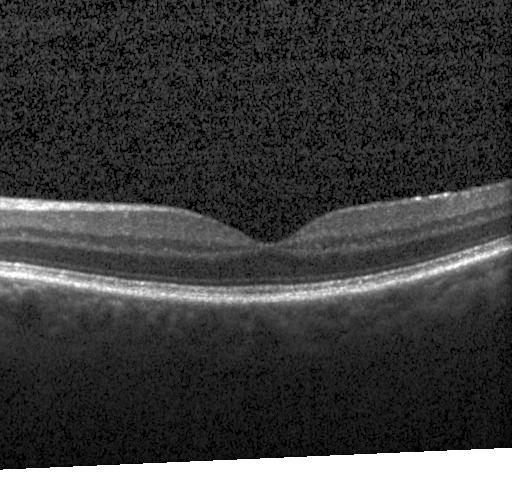

Optical coherence tomography B-scan; spectral-domain OCT. Diagnosis: no CNV, DME, or drusen.